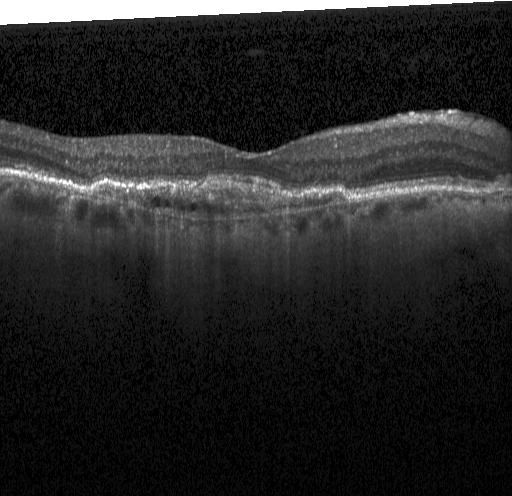
Heidelberg Spectralis OCT system · OCT line scan · through the macula · spectral-domain optical coherence tomography
Diagnosis: a choroidal neovascular membrane.